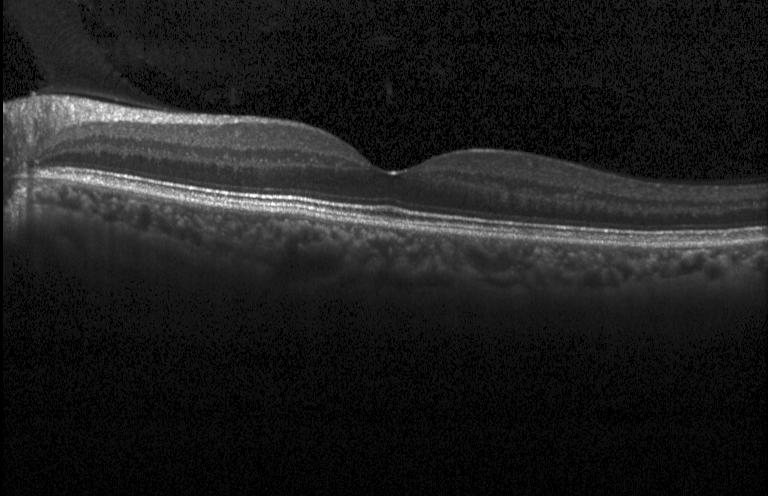 Diagnosis: no choroidal neovascularization, no diabetic macular edema, and no drusen.